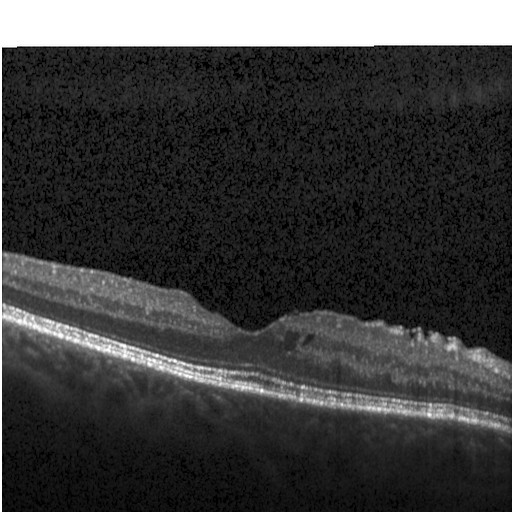

Retinal OCT cross-section. DME.